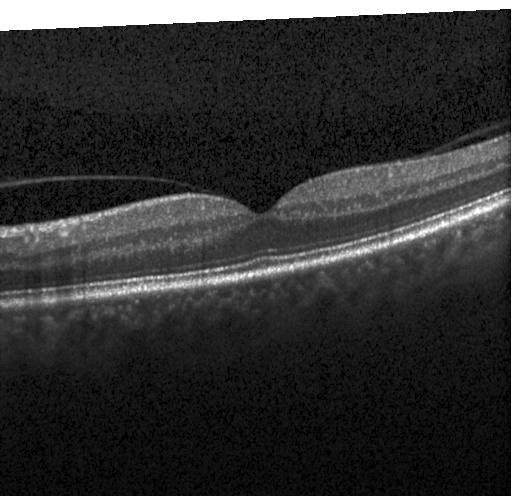 Finding: no evidence of choroidal neovascularization, diabetic macular edema, or drusen.